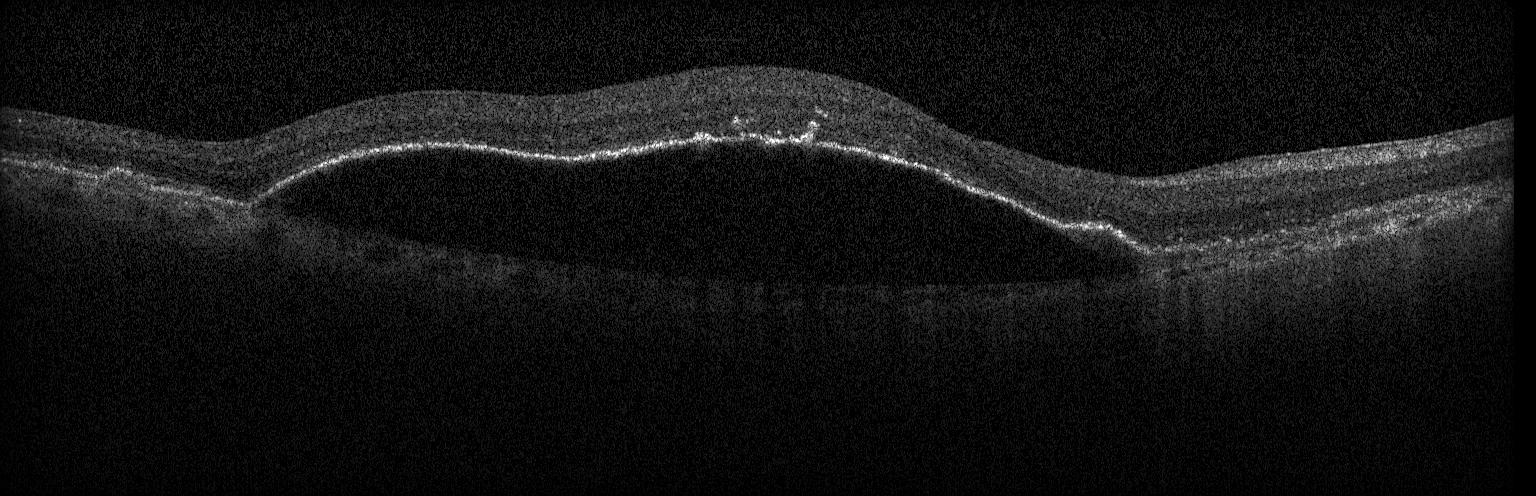 Heidelberg Spectralis. OCT line scan. Fovea-centered
Macular OCT: a choroidal neovascular membrane.